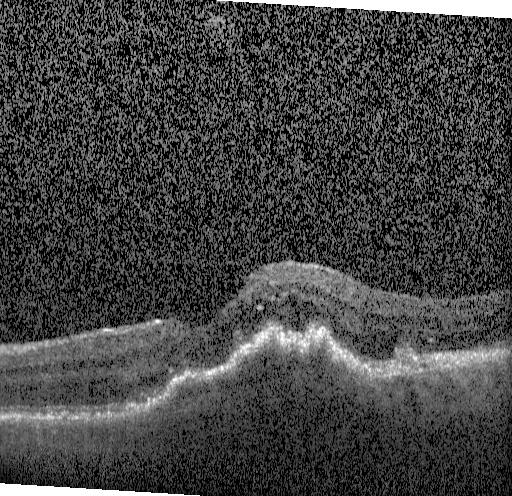 OCT line scan · spectral-domain optical coherence tomography · fovea-centered · Heidelberg Spectralis OCT system — Diagnosis: a choroidal neovascular membrane.